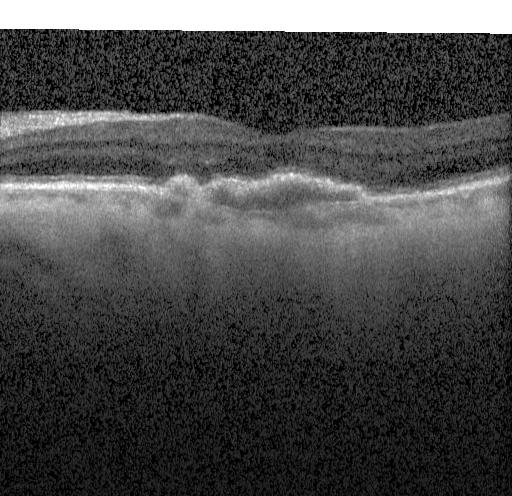
Optical coherence tomography scan. Instrument: Heidelberg Spectralis
Dx: a choroidal neovascular membrane.